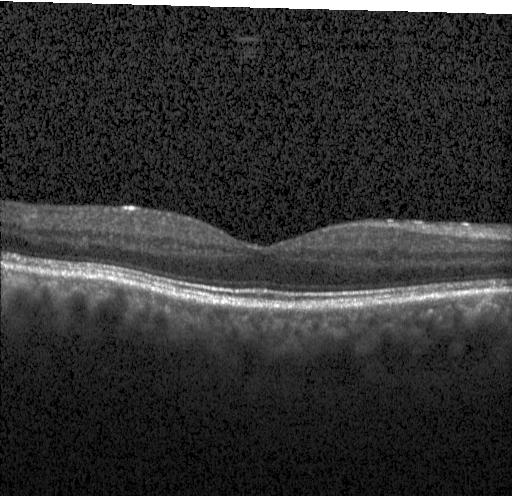
Finding: no choroidal neovascularization, diabetic macular edema, or drusen.